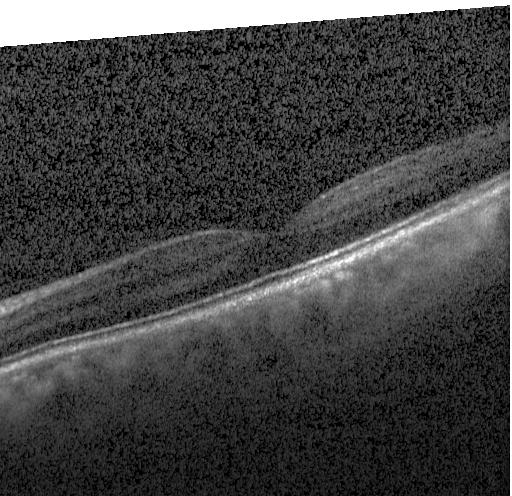

No evidence of CNV, DME, or drusen.